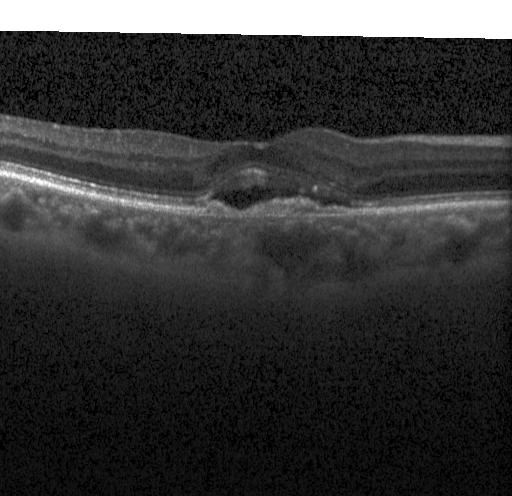
Spectral-domain optical coherence tomography · OCT B-scan · horizontal scan through the fovea
Assessment: choroidal neovascularization (CNV).